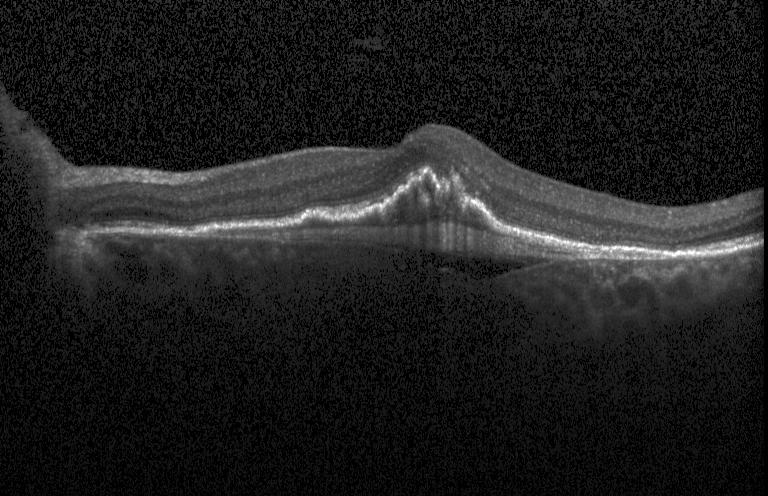

Heidelberg Spectralis OCT system. Spectral-domain optical coherence tomography. Through the macula. Retinal OCT cross-section. This B-scan demonstrates a choroidal neovascular membrane.